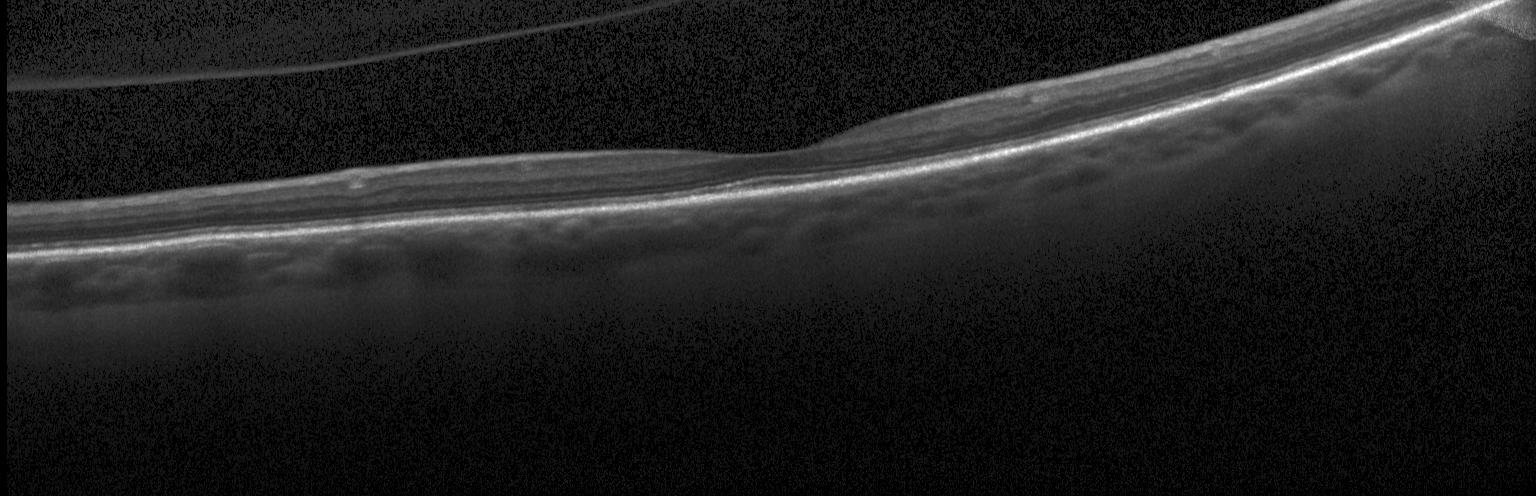

OCT line scan. Heidelberg Spectralis OCT system
Dx: neither CNV, DME, nor drusen.